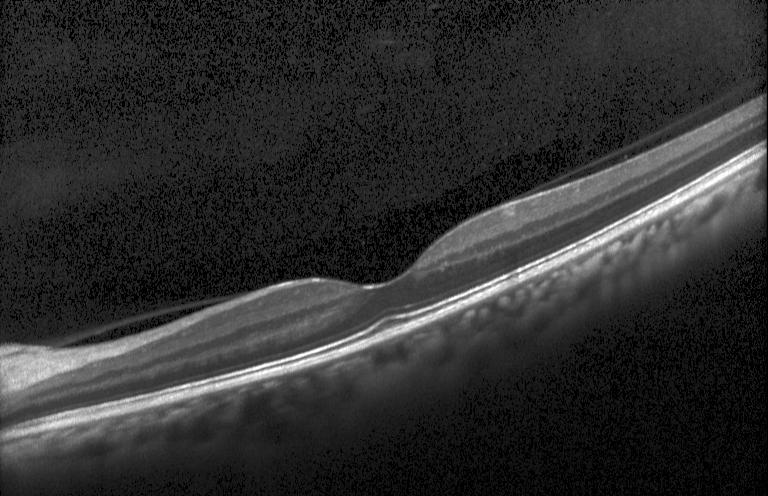 Diagnosis: no evidence of choroidal neovascularization, diabetic macular edema, or drusen.